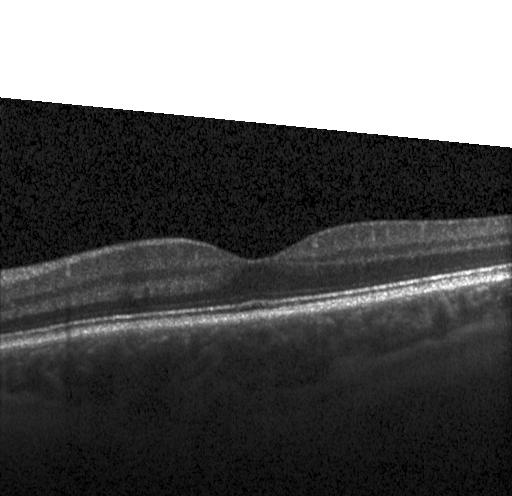 OCT line scan — Dx: neither choroidal neovascularization, diabetic macular edema, nor drusen.